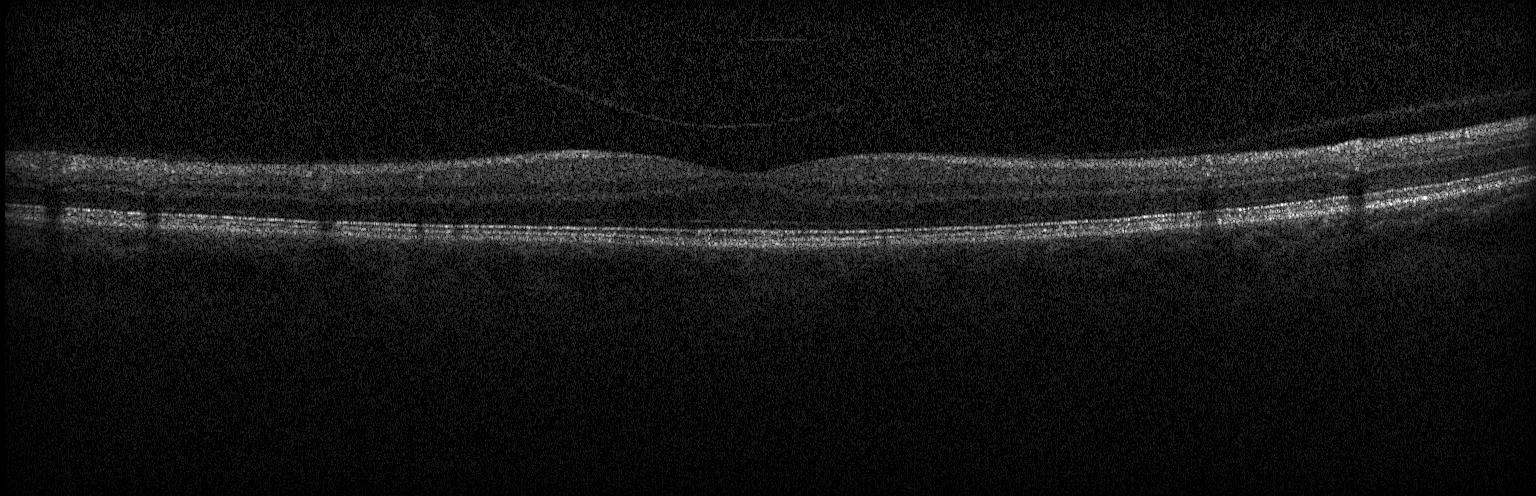 Heidelberg Spectralis OCT system; optical coherence tomography B-scan; spectral-domain OCT; fovea-centered. Impression: no choroidal neovascularization, no diabetic macular edema, and no drusen.